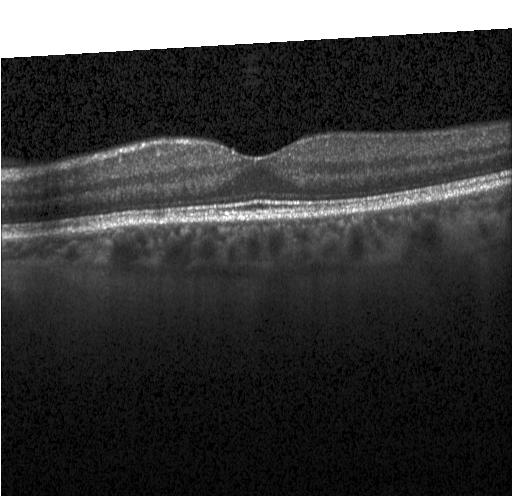
OCT line scan — Impression: no evidence of CNV, DME, or drusen.